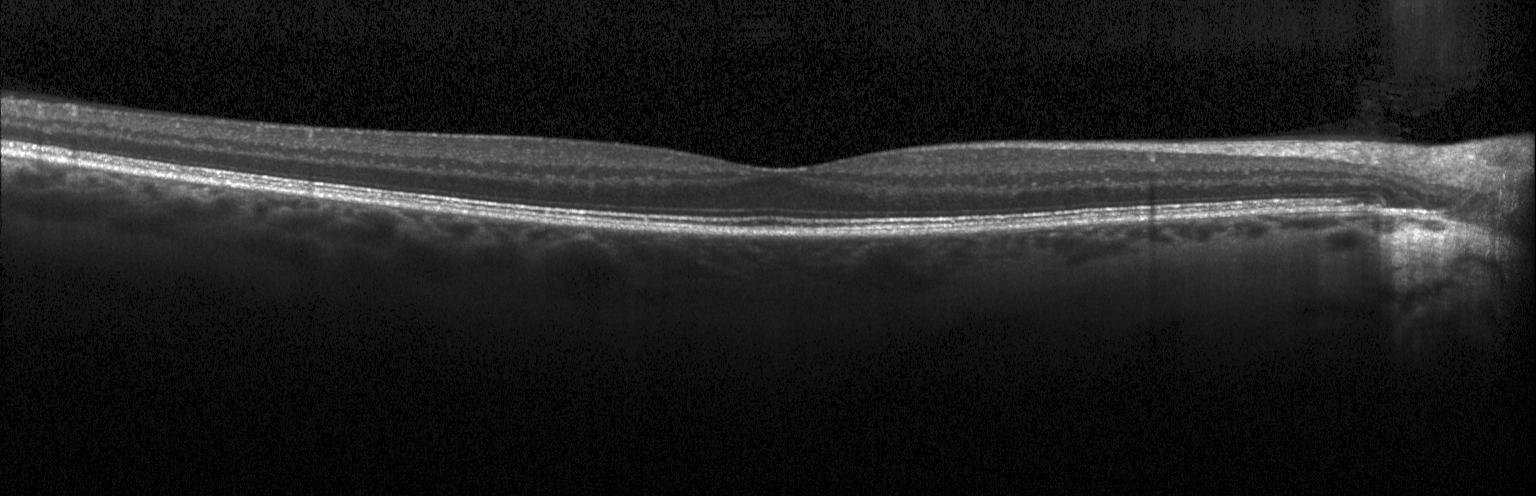 OCT B-scan
No CNV, DME, or drusen.